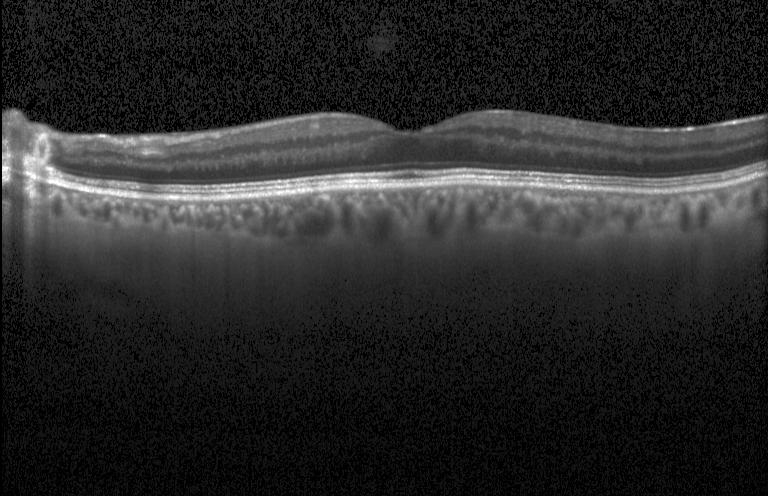

Instrument: Heidelberg Spectralis. Retinal OCT B-scan.
Impression: no evidence of choroidal neovascularization, diabetic macular edema, or drusen.